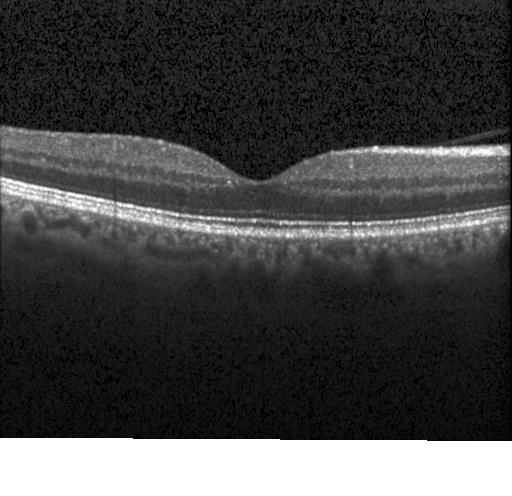

Fovea-centered, OCT B-scan, instrument: Heidelberg Spectralis
Finding: neither choroidal neovascularization, diabetic macular edema, nor drusen.